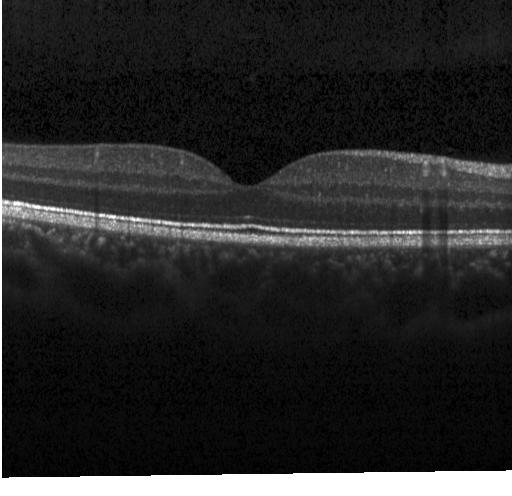
Optical coherence tomography scan. Diagnosis: no CNV, no DME, and no drusen.